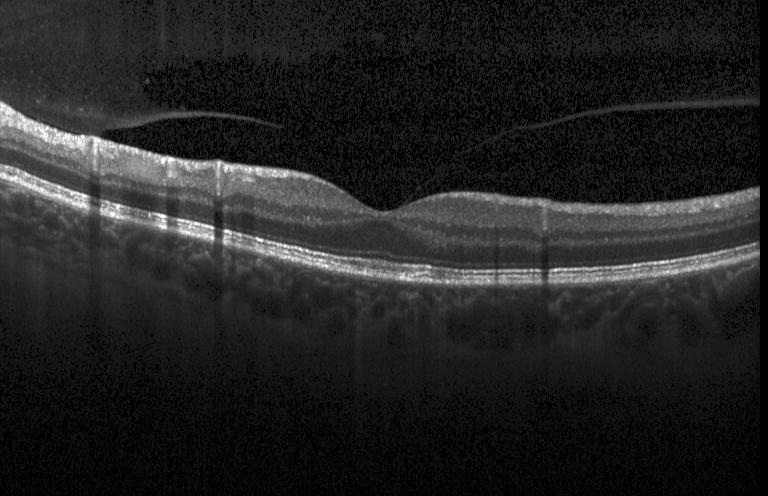

Retinal OCT cross-section. OCT finding: no evidence of CNV, DME, or drusen.